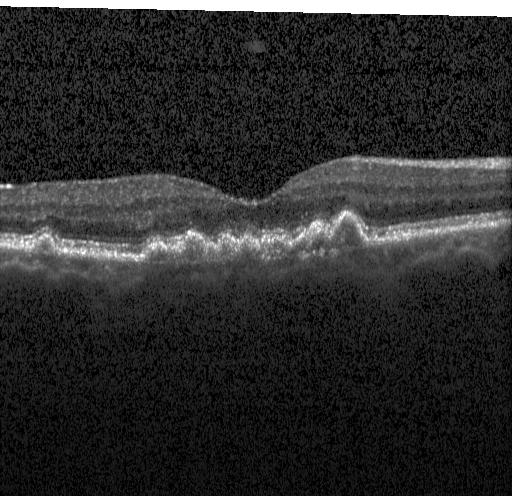

Retinal OCT cross-section — Impression: multiple drusen.